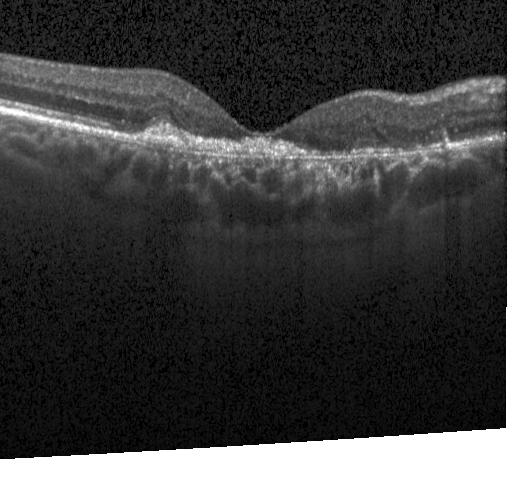
Optical coherence tomography B-scan; horizontal scan through the fovea; spectral-domain OCT; instrument: Heidelberg Spectralis — Macular OCT: choroidal neovascularization (CNV).